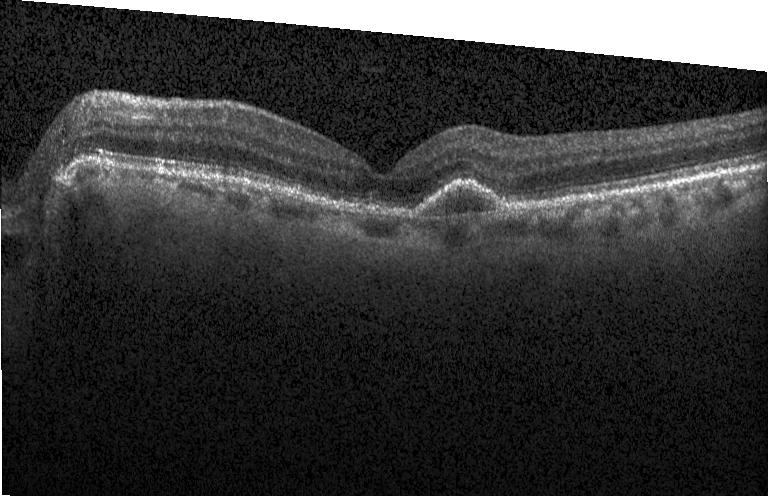
The scan shows a choroidal neovascular membrane.